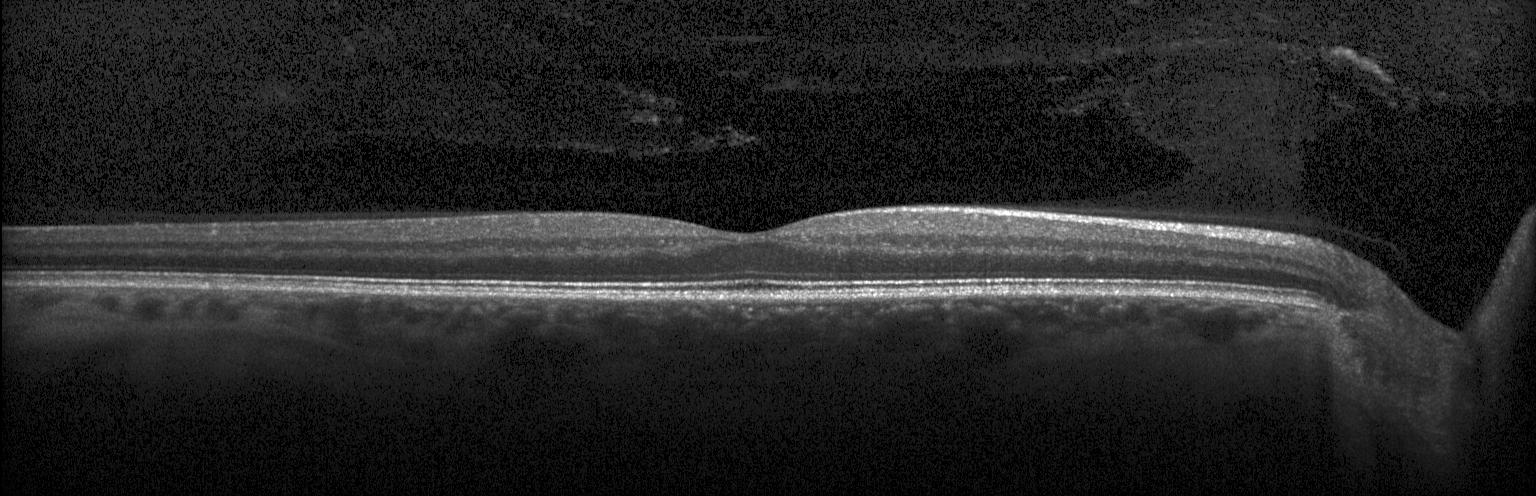

Diagnosis: no evidence of choroidal neovascularization, diabetic macular edema, or drusen.